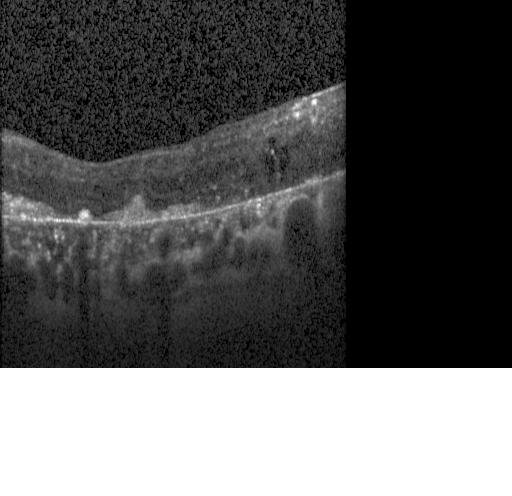 The scan shows CNV.